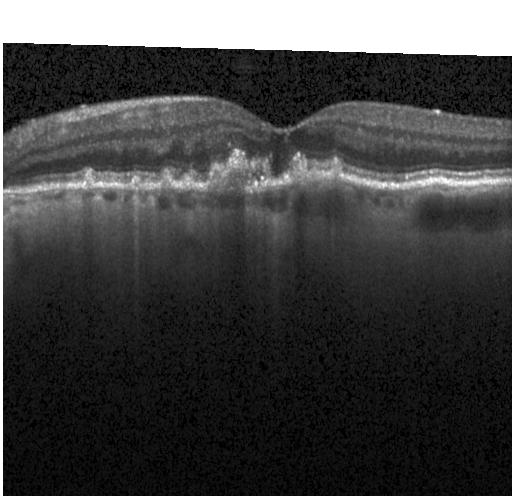 This B-scan demonstrates choroidal neovascularization (CNV).